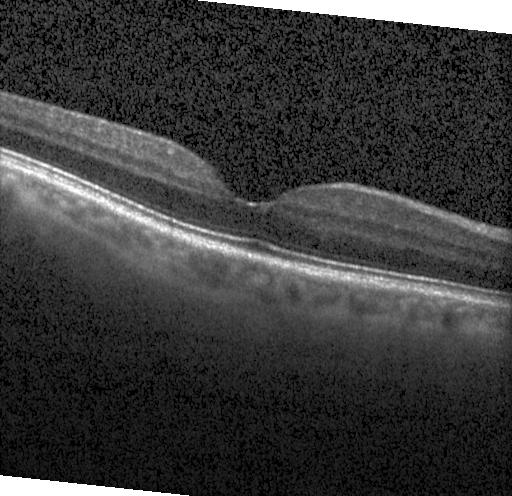
OCT line scan. Diagnosis: no evidence of CNV, DME, or drusen.